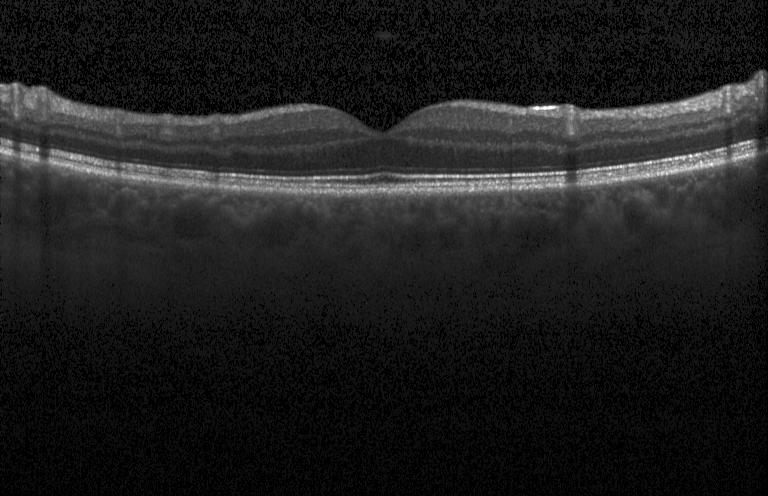
Fovea-centered, acquired on a Heidelberg Spectralis, optical coherence tomography B-scan, spectral-domain OCT — Macular OCT: neither CNV, DME, nor drusen.